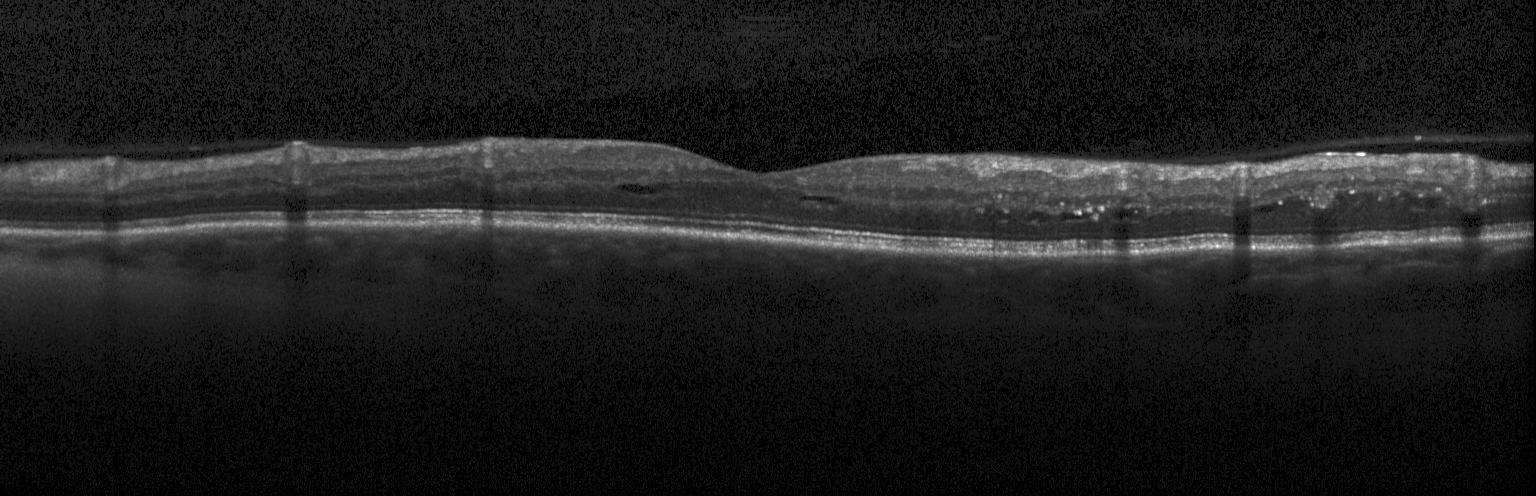

Spectral-domain optical coherence tomography · OCT B-scan · fovea-centered · Heidelberg Spectralis OCT system — Impression: diabetic macular edema.